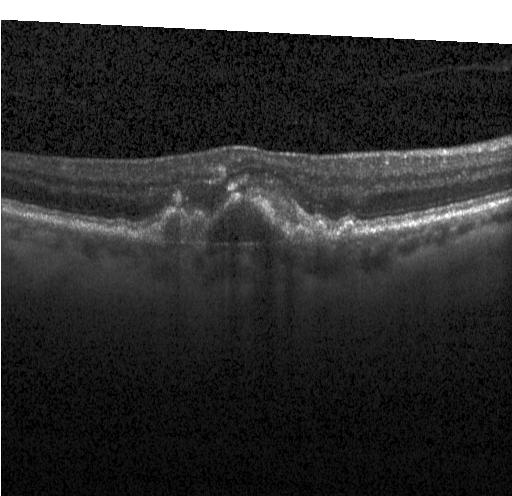

Retinal OCT cross-section. Spectral-domain optical coherence tomography. Horizontal scan through the fovea. Heidelberg Spectralis.
Finding: choroidal neovascularization (CNV).